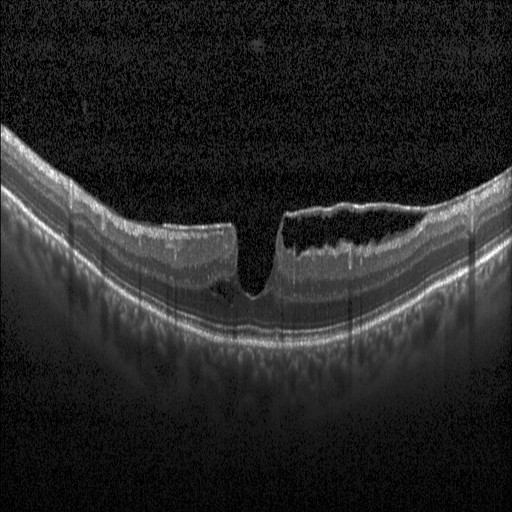 Optical coherence tomography scan; SD-OCT. OCT finding: DME.